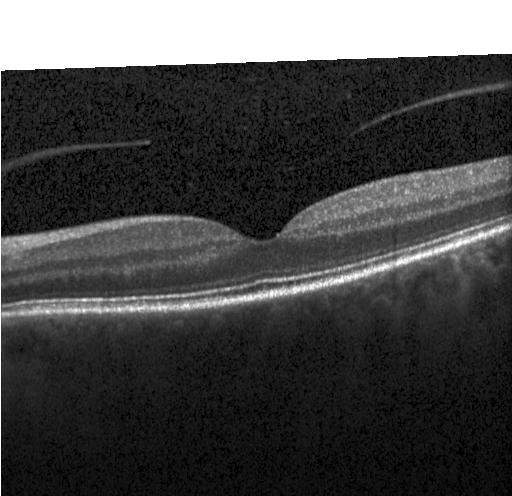
Spectral-domain OCT; OCT B-scan
Finding: no CNV, DME, or drusen.